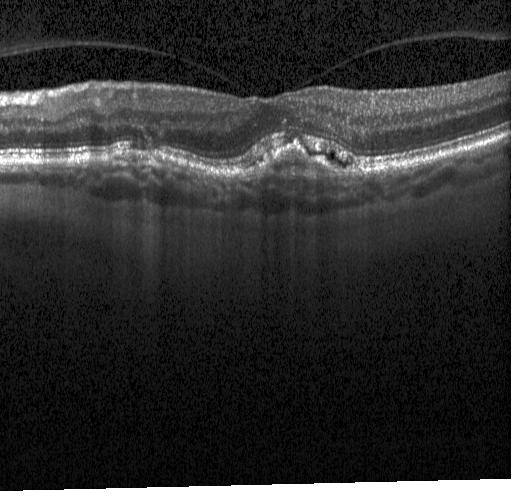
The scan shows a choroidal neovascular membrane.